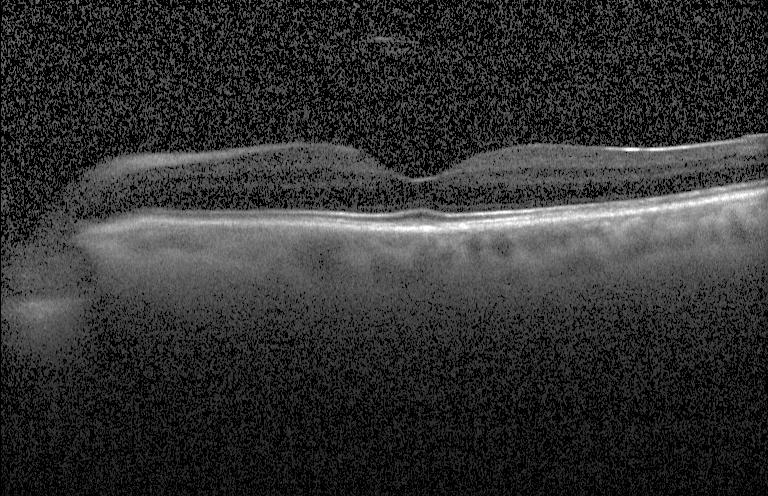
Macular scan, spectral-domain optical coherence tomography, retinal OCT B-scan — This B-scan demonstrates no choroidal neovascularization, diabetic macular edema, or drusen.